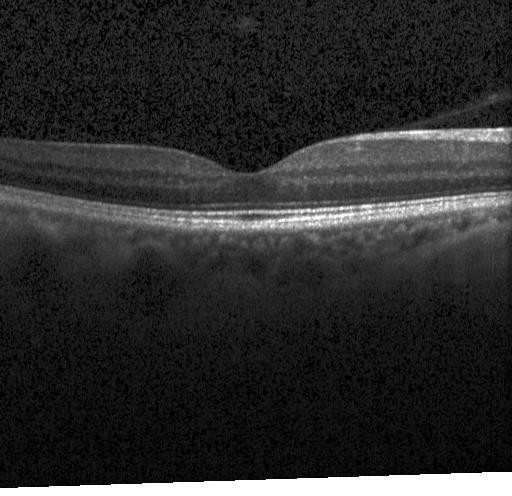 Optical coherence tomography scan. Heidelberg Spectralis OCT system. Diagnosis: neither choroidal neovascularization, diabetic macular edema, nor drusen.